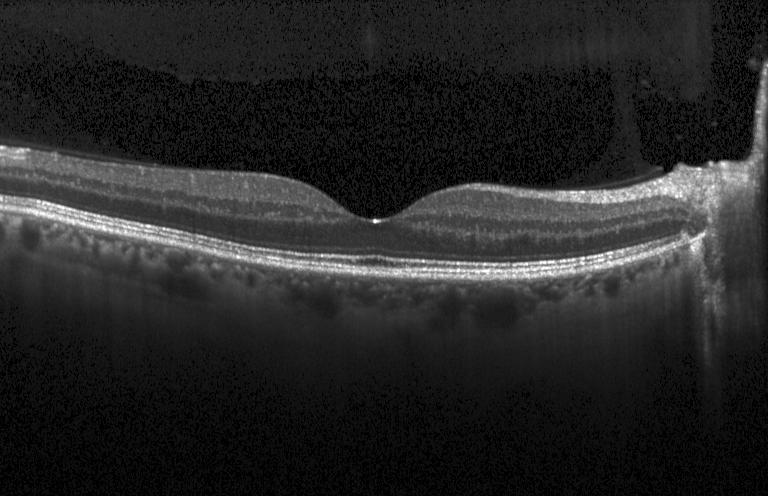

OCT B-scan showing no CNV, no DME, and no drusen.